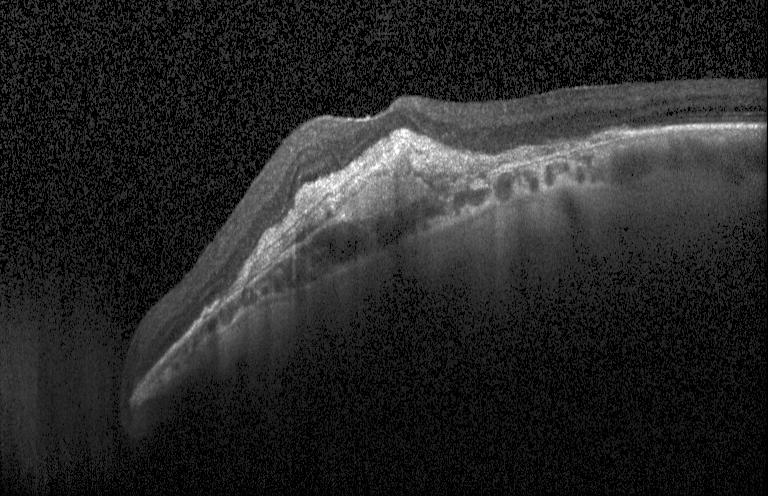 Retinal OCT B-scan; horizontal scan through the fovea; spectral-domain OCT — This B-scan demonstrates a choroidal neovascular membrane.